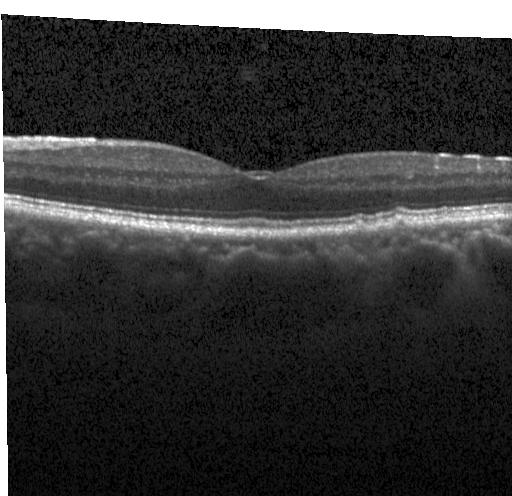
Finding: multiple drusen.